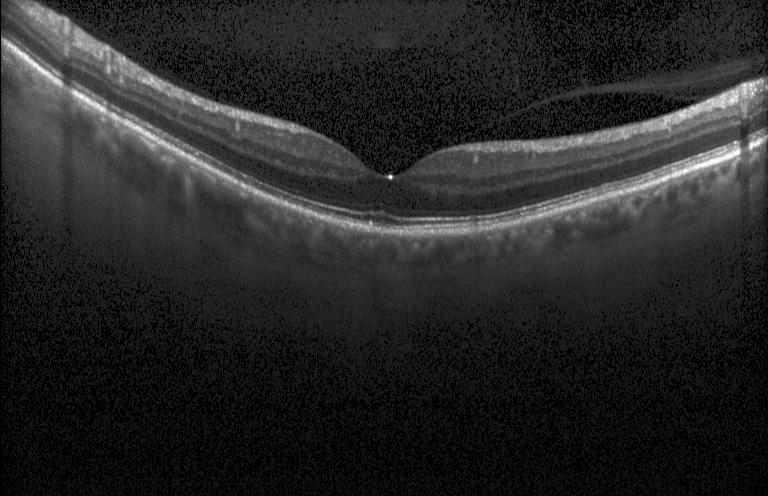 Finding: neither choroidal neovascularization, diabetic macular edema, nor drusen.